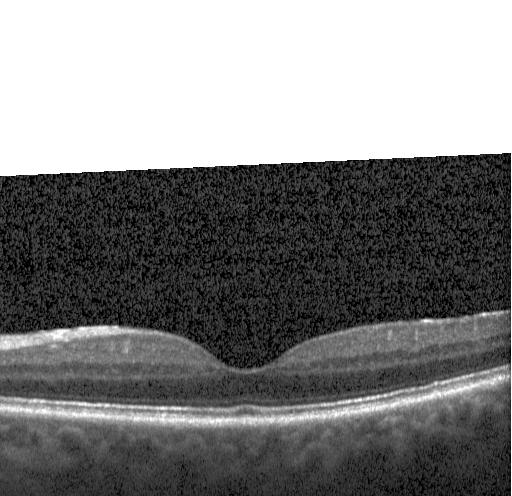
OCT line scan. Spectral-domain OCT. Instrument: Heidelberg Spectralis — Diagnosis: no choroidal neovascularization, diabetic macular edema, or drusen.